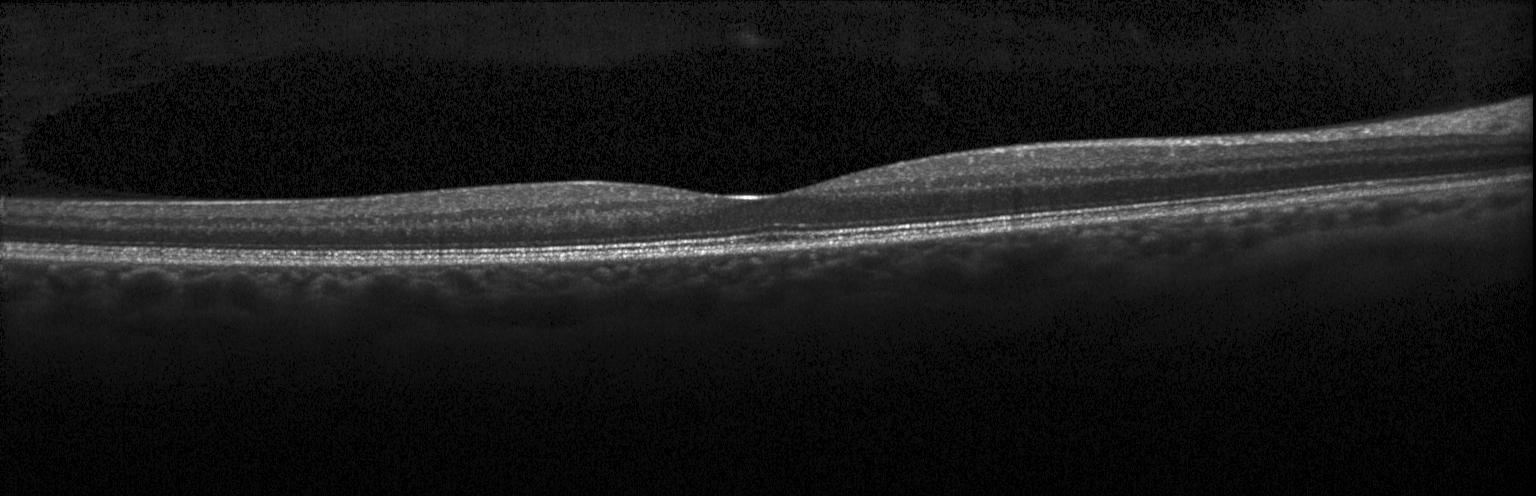

No choroidal neovascularization, no diabetic macular edema, and no drusen.